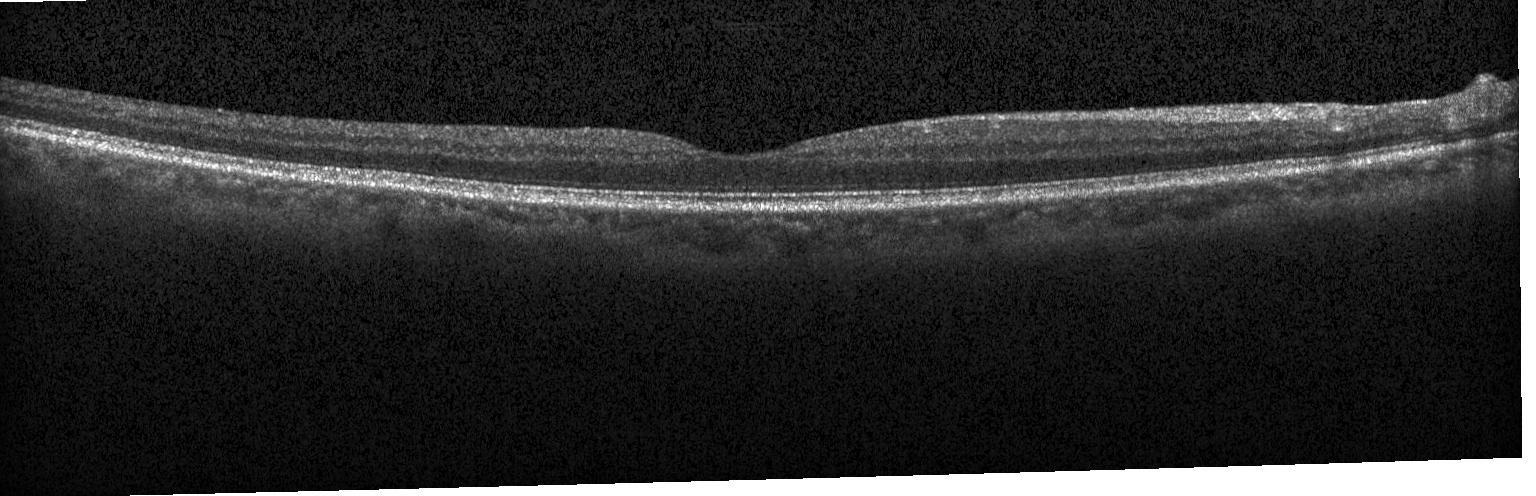 Macular scan, retinal OCT cross-section. This B-scan demonstrates neither choroidal neovascularization, diabetic macular edema, nor drusen.